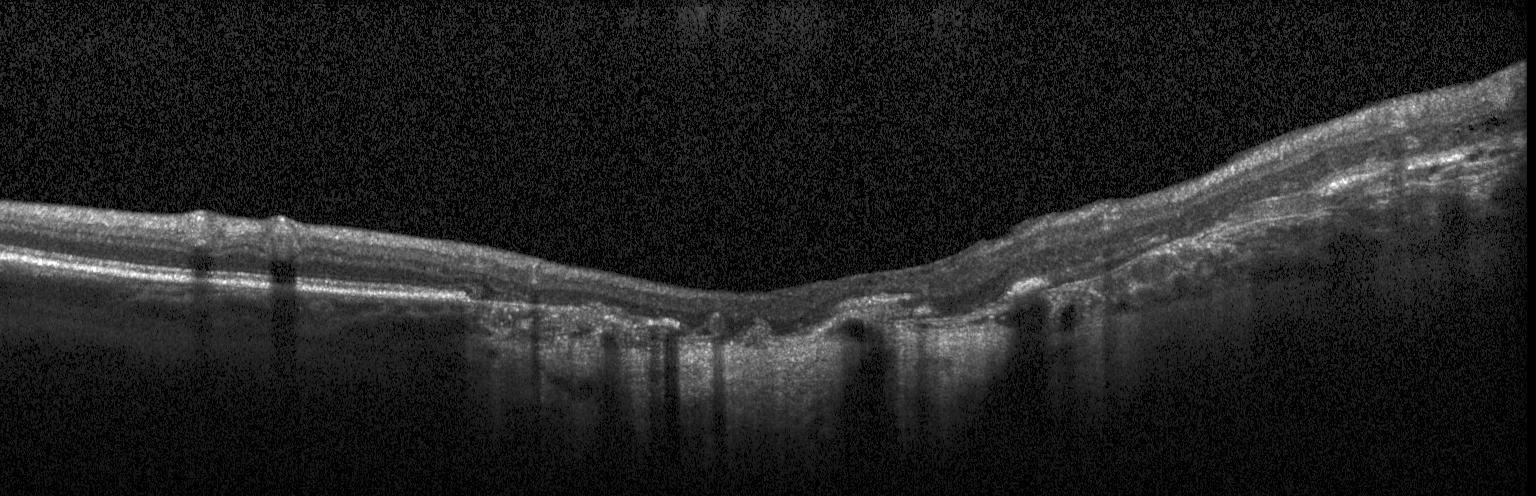

The scan shows CNV.